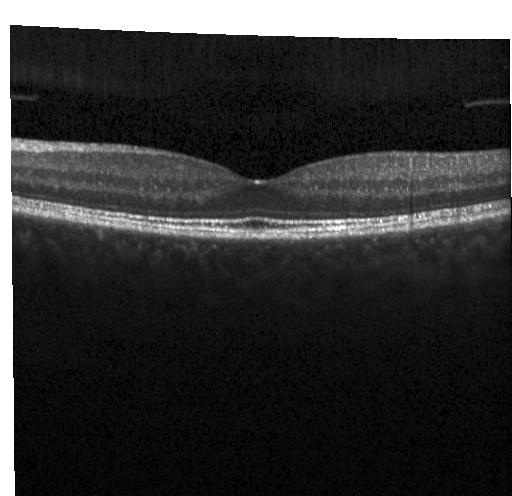 Acquired on a Heidelberg Spectralis · spectral-domain optical coherence tomography · optical coherence tomography B-scan. Diagnosis: no choroidal neovascularization, diabetic macular edema, or drusen.